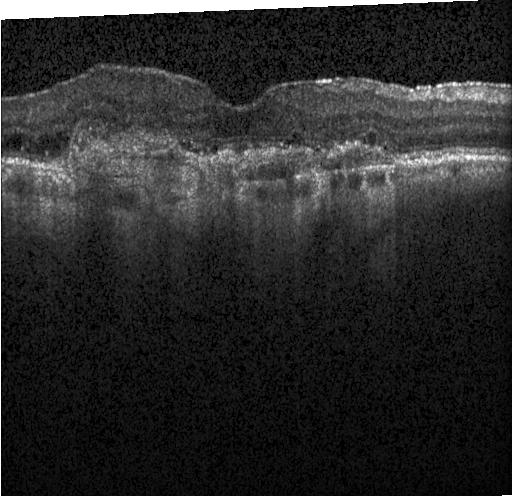 Instrument: Heidelberg Spectralis · spectral-domain OCT · horizontal scan through the fovea · retinal OCT cross-section
Dx: a choroidal neovascular membrane.